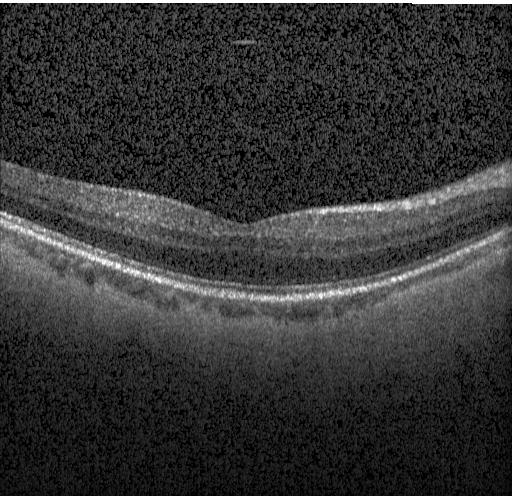 Optical coherence tomography scan; Heidelberg Spectralis OCT system; centered on the fovea.
Impression: no evidence of choroidal neovascularization, diabetic macular edema, or drusen.